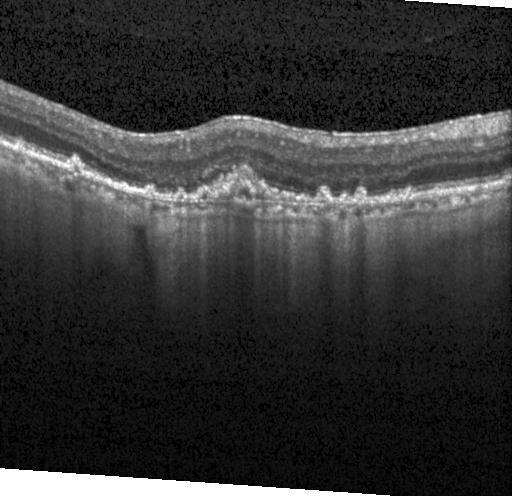

A choroidal neovascular membrane.